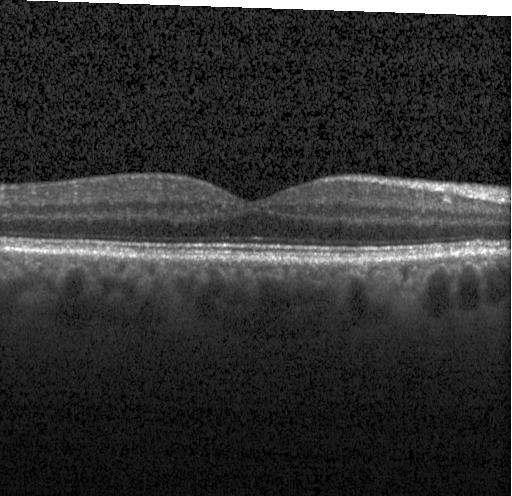

Macular OCT: no evidence of CNV, DME, or drusen.